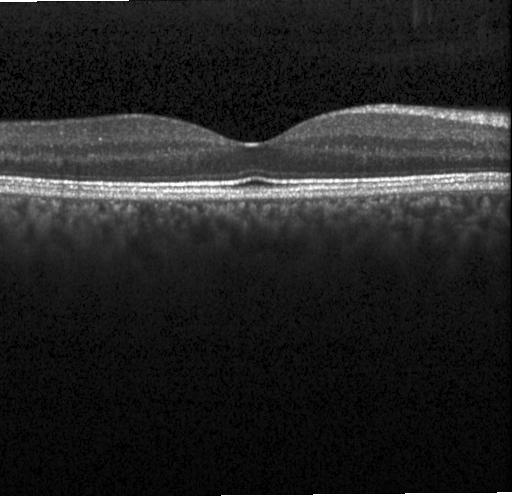

Spectral-domain optical coherence tomography · OCT B-scan · acquired on a Heidelberg Spectralis. Diagnosis: no evidence of choroidal neovascularization, diabetic macular edema, or drusen.